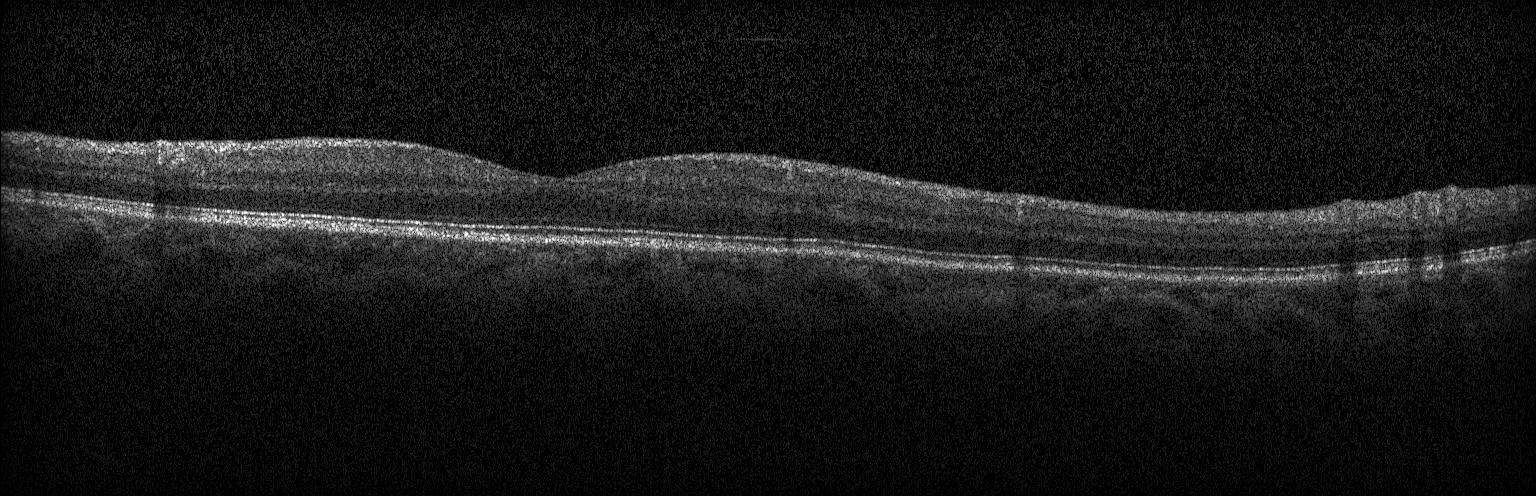

OCT B-scan showing no choroidal neovascularization, no diabetic macular edema, and no drusen.